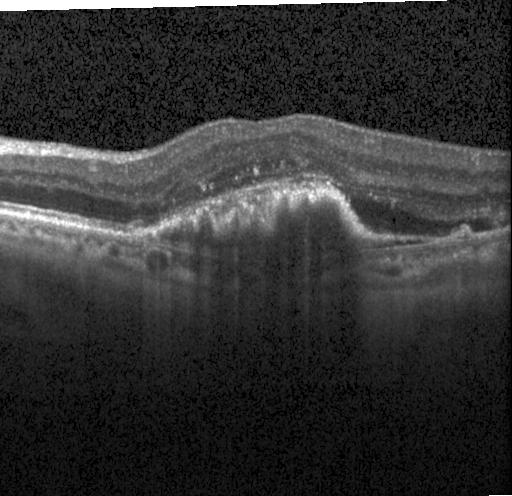 OCT line scan.
The scan shows a choroidal neovascular membrane.